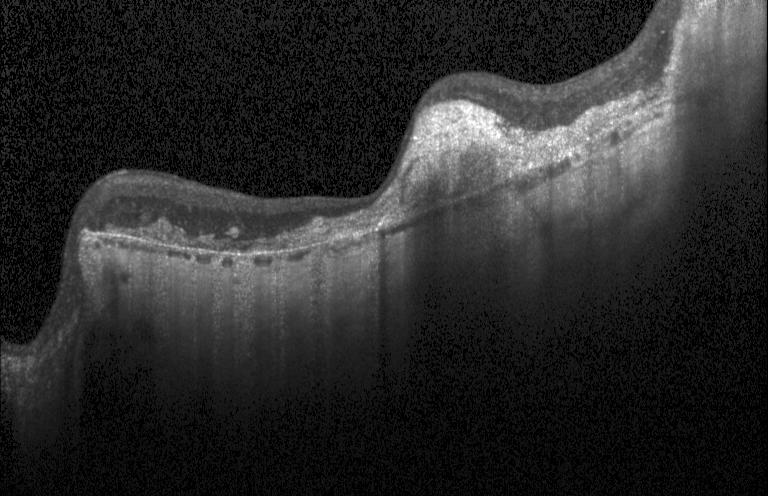 Impression: a choroidal neovascular membrane.